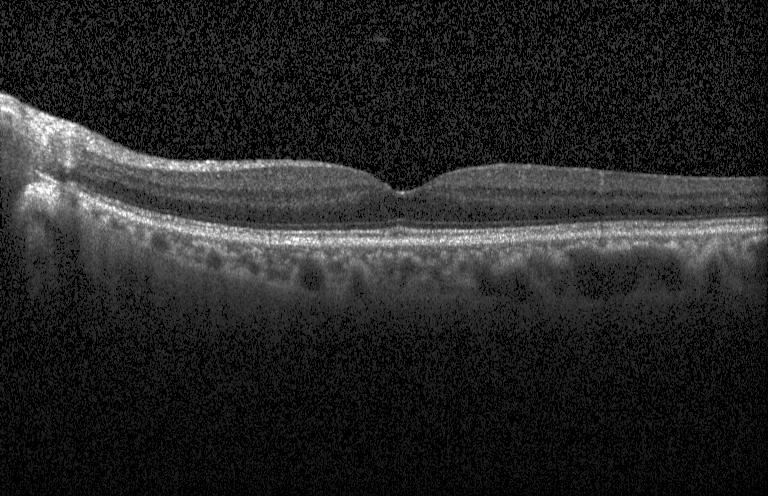
Optical coherence tomography scan, acquired on a Heidelberg Spectralis, through the macula, spectral-domain optical coherence tomography
This B-scan demonstrates neither choroidal neovascularization, diabetic macular edema, nor drusen.